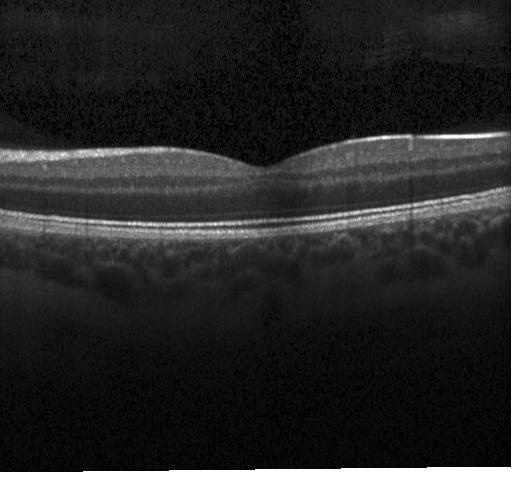

Spectral-domain optical coherence tomography; centered on the fovea; retinal OCT B-scan.
Diagnosis: no choroidal neovascularization, no diabetic macular edema, and no drusen.